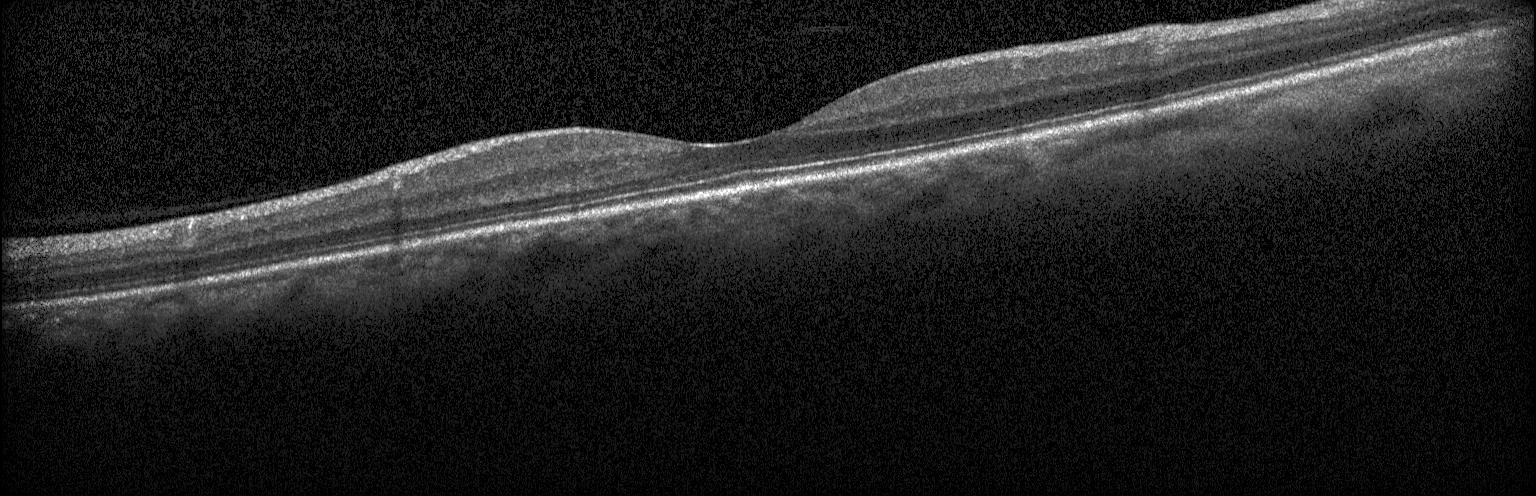

OCT finding: no evidence of choroidal neovascularization, diabetic macular edema, or drusen.